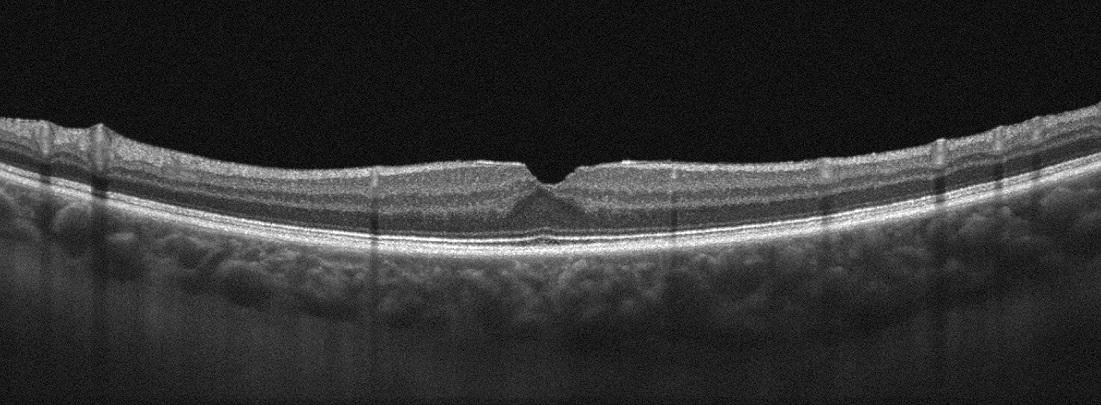

OCT finding: epiretinal membrane (ERM).